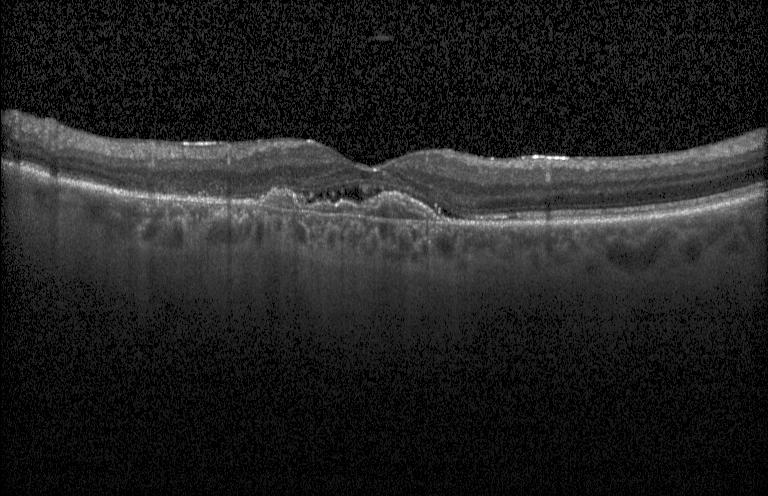
Macular OCT demonstrating CNV.